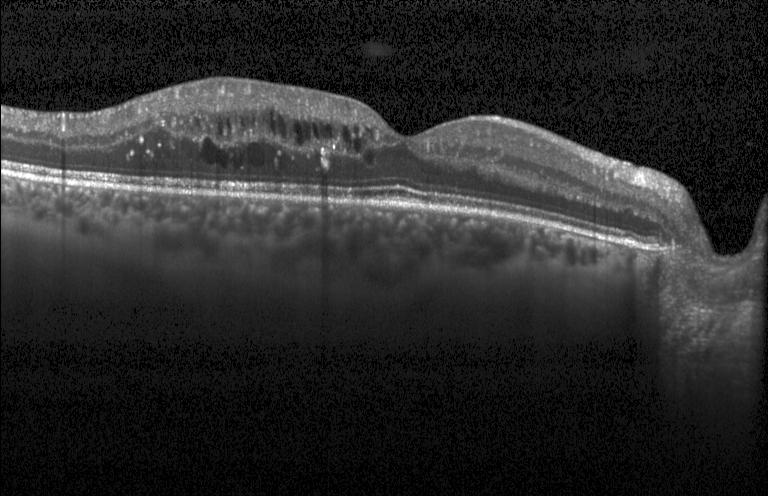 Retinal OCT cross-section showing DME.